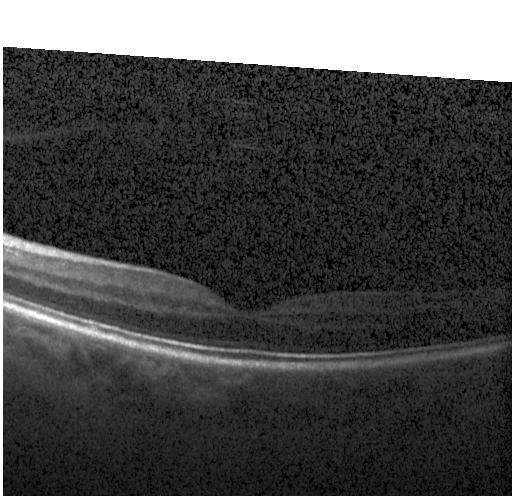 Retinal OCT cross-section — Impression: no CNV, no DME, and no drusen.